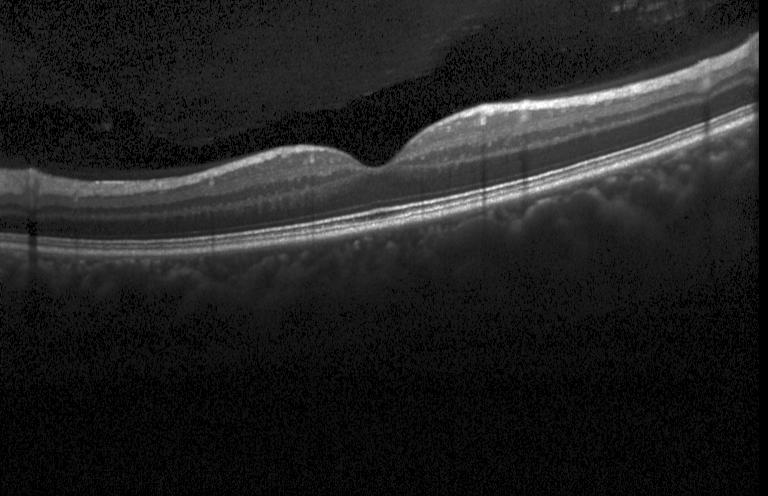
Optical coherence tomography B-scan
Impression: no evidence of CNV, DME, or drusen.